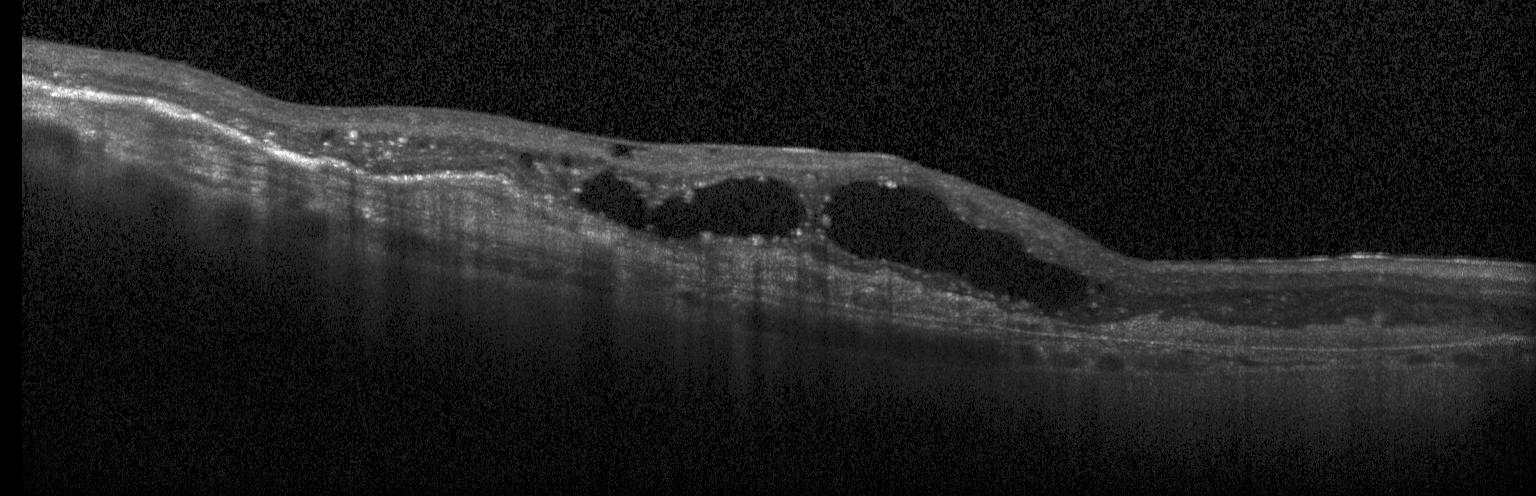 Optical coherence tomography scan. Acquired on a Heidelberg Spectralis — Finding: a choroidal neovascular membrane.